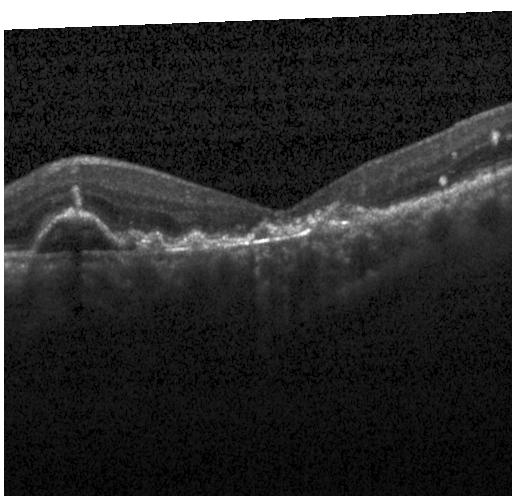

Spectral-domain OCT. Acquired on a Heidelberg Spectralis. Macular scan. Optical coherence tomography B-scan
Impression: CNV.